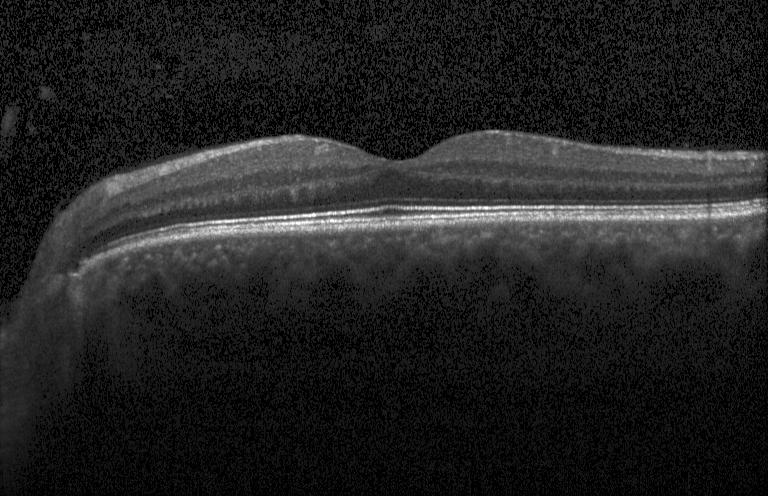 SD-OCT, Heidelberg Spectralis OCT system, OCT B-scan. Finding: no choroidal neovascularization, diabetic macular edema, or drusen.